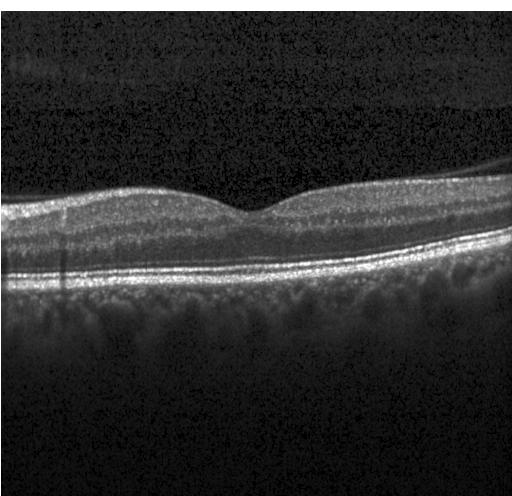
Macular OCT demonstrating no CNV, DME, or drusen.